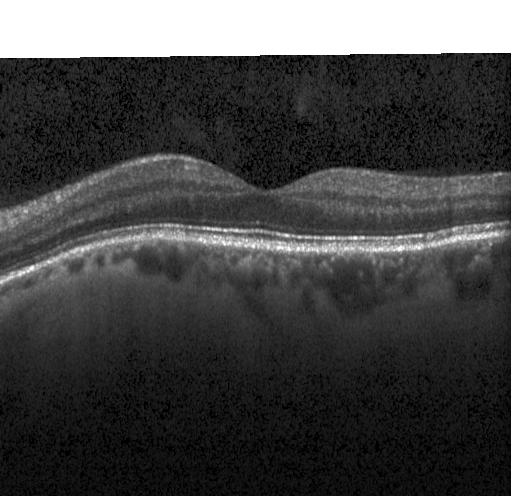
Fovea-centered. Heidelberg Spectralis. OCT line scan. Spectral-domain optical coherence tomography
Impression: no choroidal neovascularization, diabetic macular edema, or drusen.